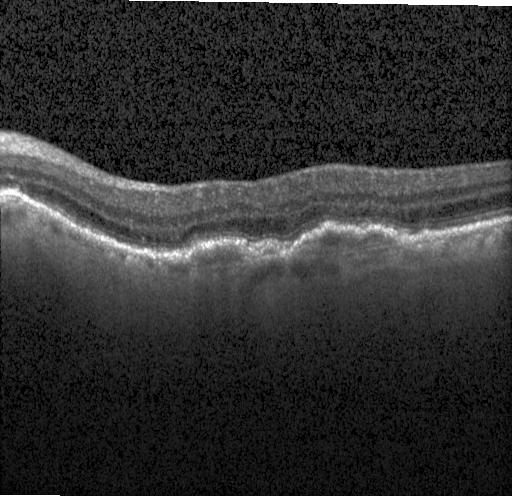
Impression: a choroidal neovascular membrane.